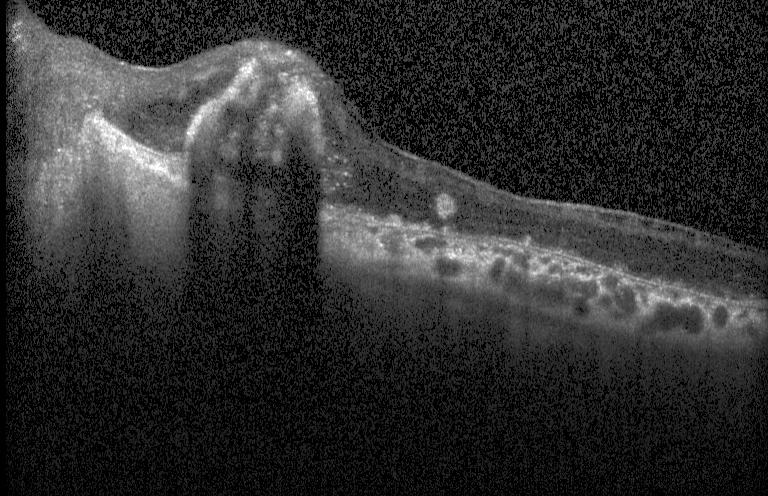
Horizontal scan through the fovea · Heidelberg Spectralis · retinal OCT cross-section. This B-scan demonstrates a choroidal neovascular membrane.